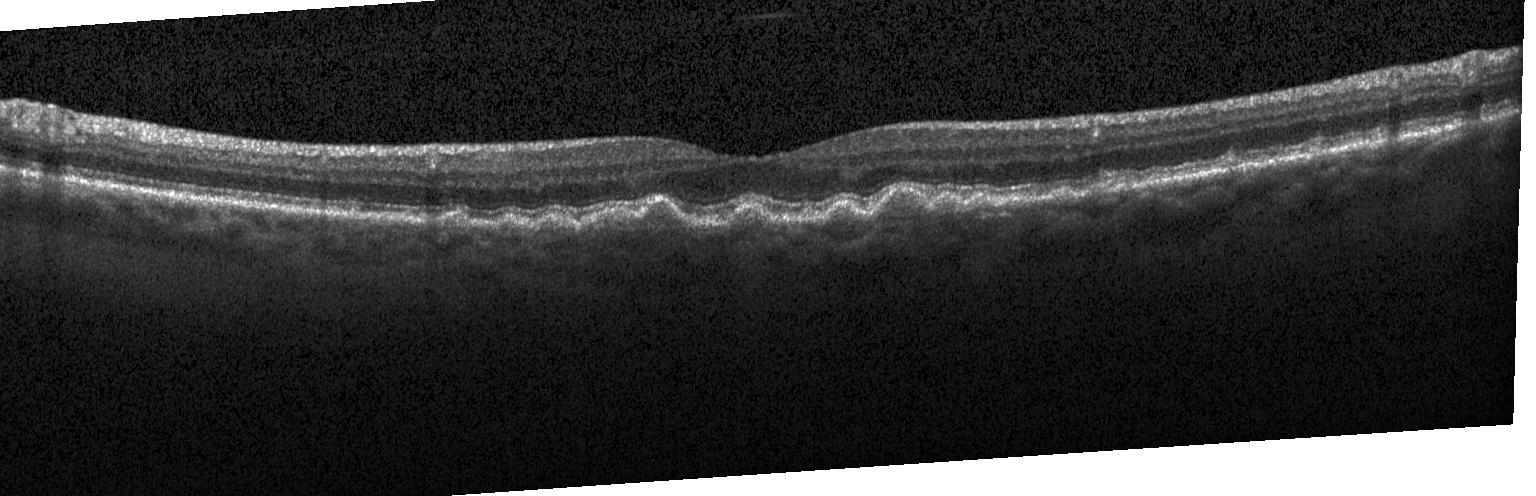 Horizontal scan through the fovea; OCT line scan; SD-OCT. Multiple drusen.